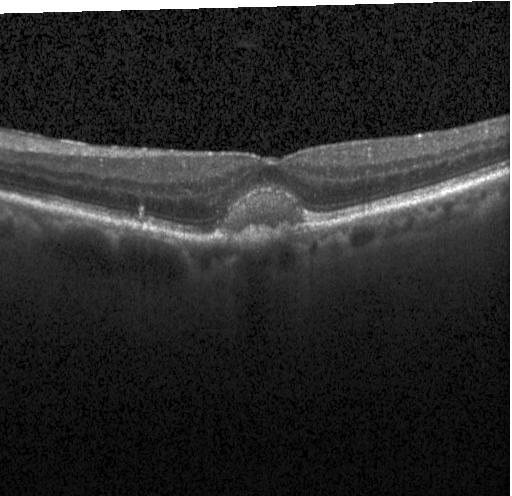
Retinal OCT cross-section
Dx: a choroidal neovascular membrane.